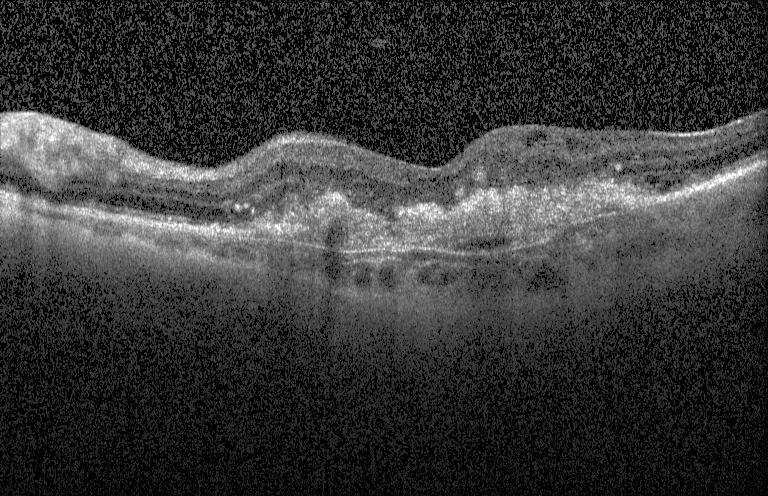

Retinal OCT cross-section; macular scan; instrument: Heidelberg Spectralis; spectral-domain optical coherence tomography.
Finding: choroidal neovascularization (CNV).